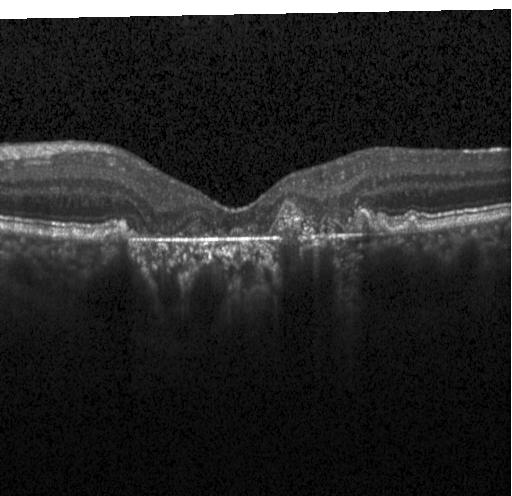
Retinal OCT cross-section. Horizontal scan through the fovea
Choroidal neovascularization (CNV).